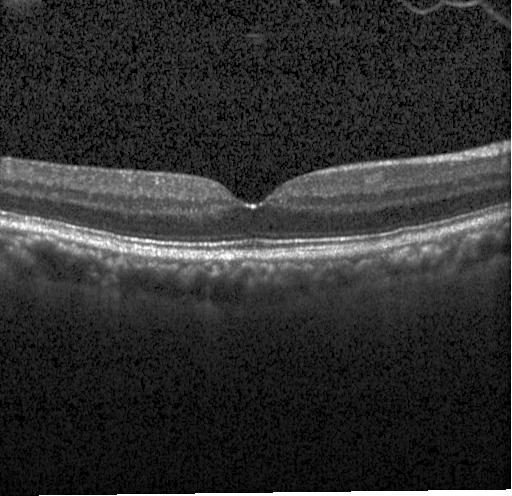
Spectral-domain optical coherence tomography, optical coherence tomography B-scan — Diagnosis: no evidence of choroidal neovascularization, diabetic macular edema, or drusen.